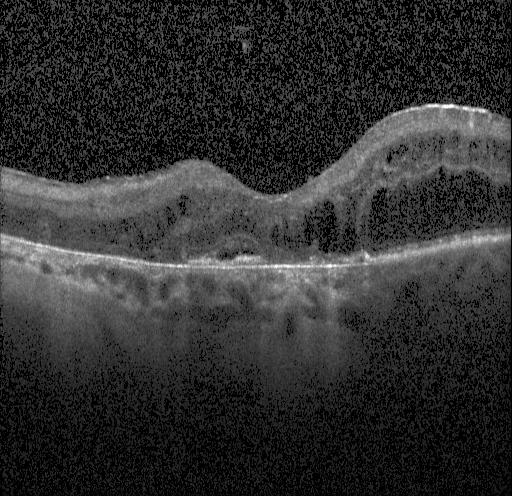

OCT line scan. Macular OCT: a choroidal neovascular membrane.